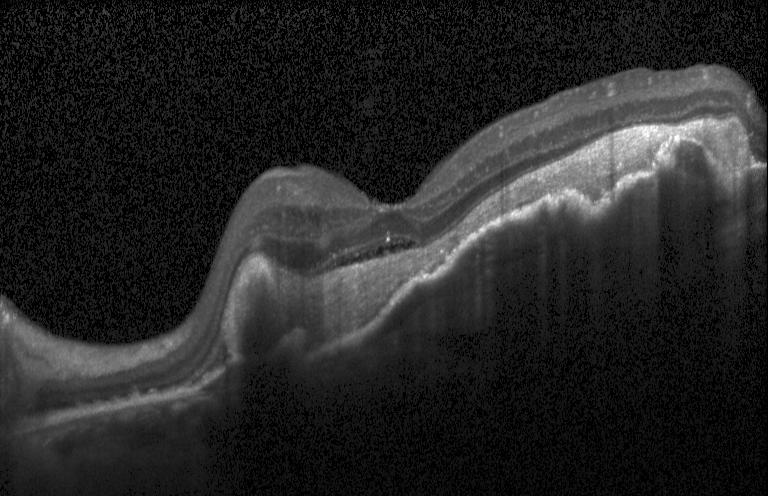 Optical coherence tomography B-scan
The scan shows a choroidal neovascular membrane.